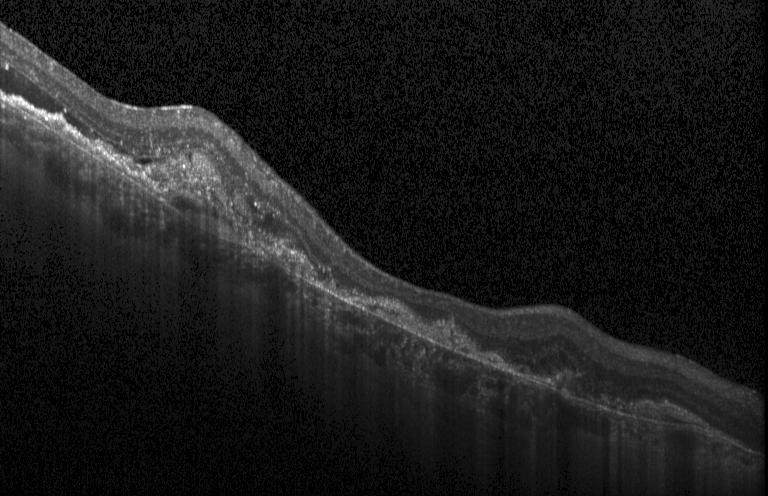
OCT finding: choroidal neovascularization.